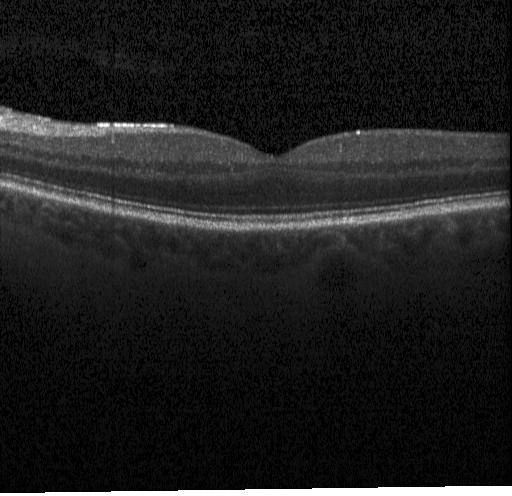 Impression: no choroidal neovascularization, no diabetic macular edema, and no drusen.